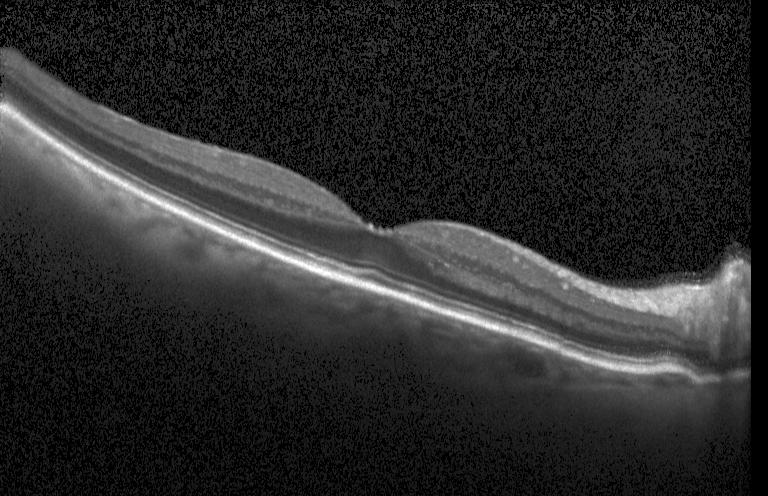

Spectral-domain OCT B-scan: no choroidal neovascularization, diabetic macular edema, or drusen.